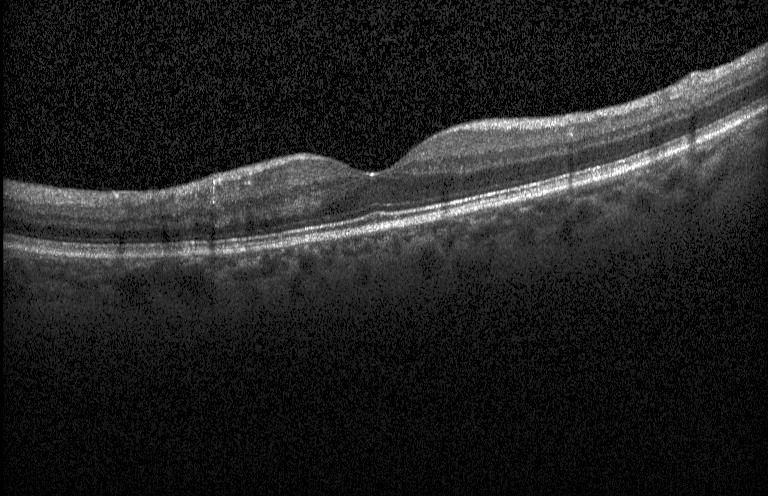

Retinal OCT cross-section.
This B-scan demonstrates neither CNV, DME, nor drusen.